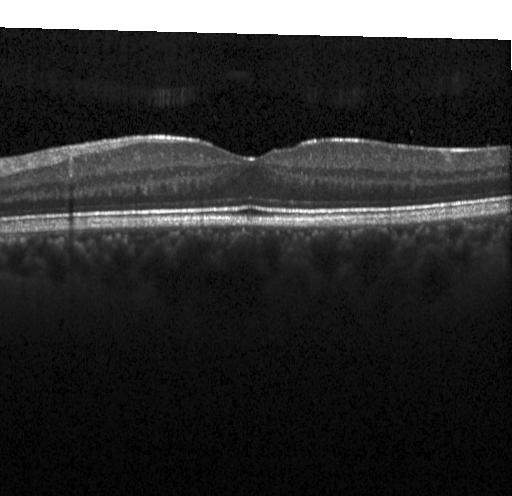
Diagnosis: no evidence of CNV, DME, or drusen.